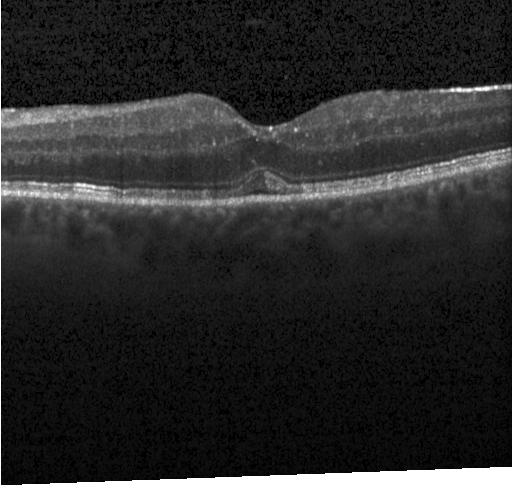
SD-OCT · macular scan · optical coherence tomography B-scan · instrument: Heidelberg Spectralis. Dx: diabetic macular edema (DME).